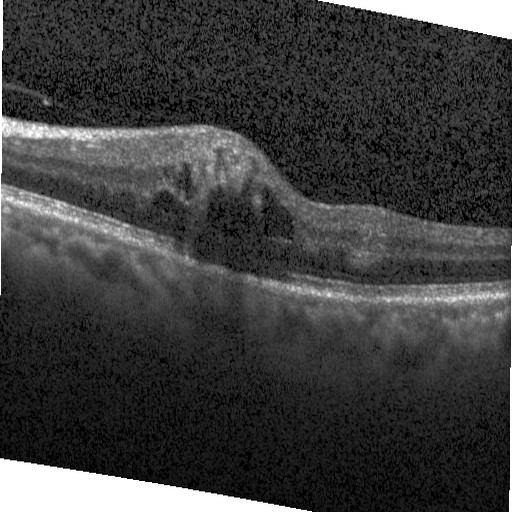
Horizontal scan through the fovea; Heidelberg Spectralis OCT system; SD-OCT; OCT line scan — This B-scan demonstrates DME.